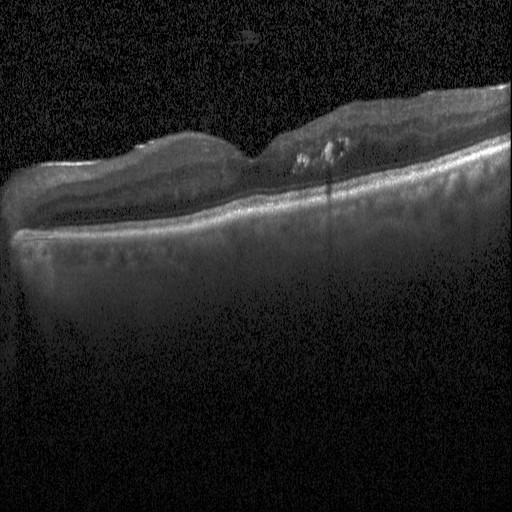

OCT B-scan · centered on the fovea · spectral-domain optical coherence tomography · acquired on a Heidelberg Spectralis. Diagnosis: diabetic macular edema (DME).